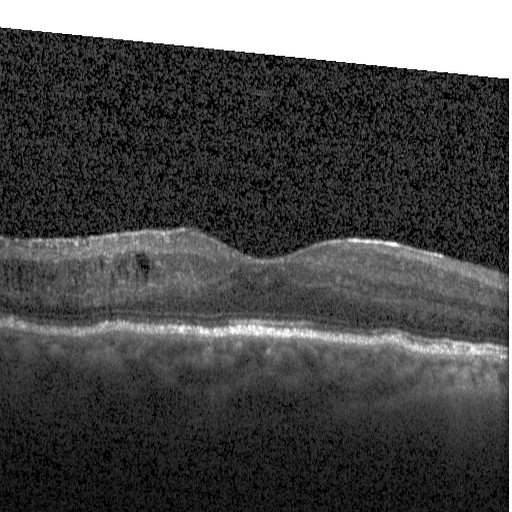
Spectral-domain OCT. OCT line scan. Assessment: DME.